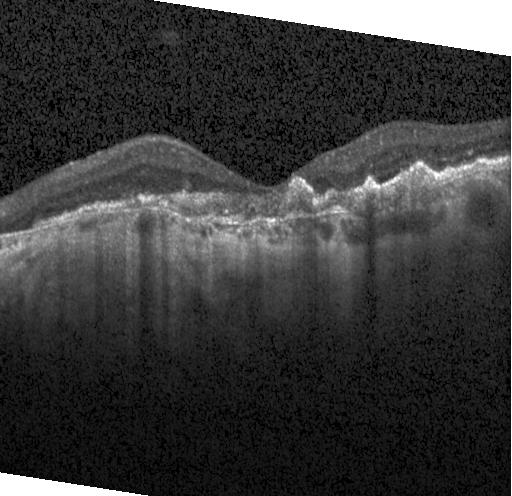

Retinal OCT cross-section · fovea-centered · spectral-domain OCT
Impression: choroidal neovascularization (CNV).